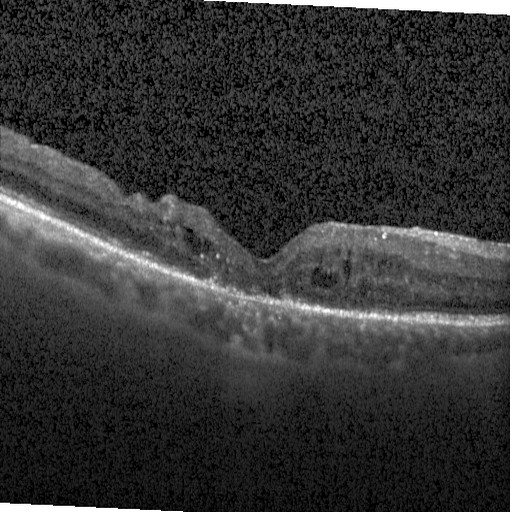

OCT line scan; horizontal scan through the fovea; instrument: Heidelberg Spectralis; spectral-domain optical coherence tomography.
Assessment: DME.